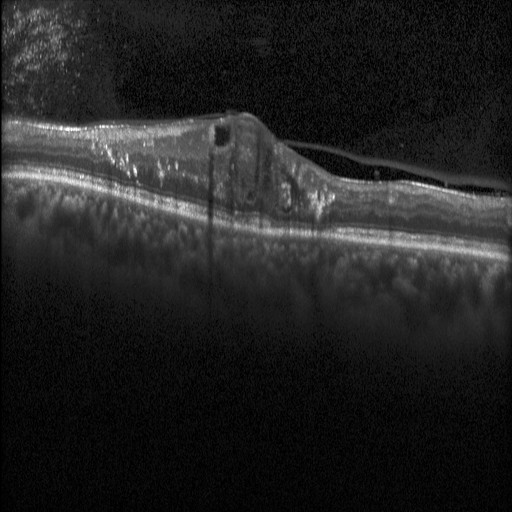 Diagnosis: diabetic macular edema.